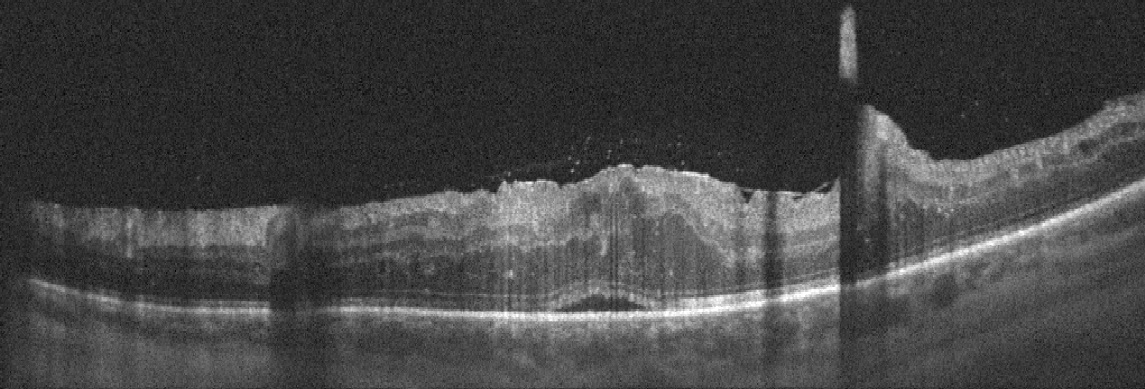
Finding: diabetic macular edema.